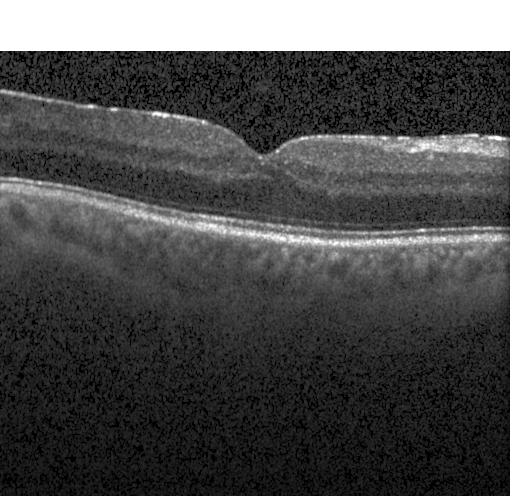
OCT finding: no choroidal neovascularization, diabetic macular edema, or drusen.